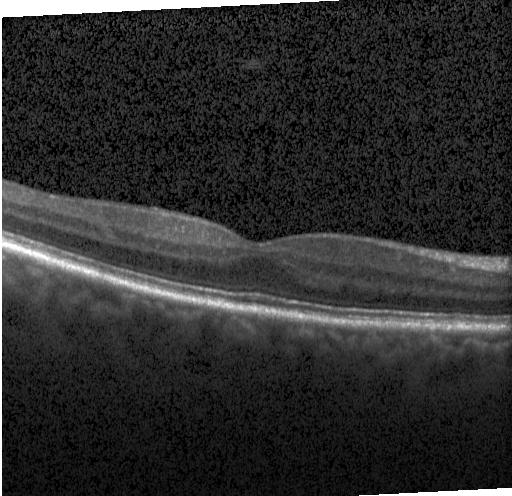
Macular OCT: neither choroidal neovascularization, diabetic macular edema, nor drusen.